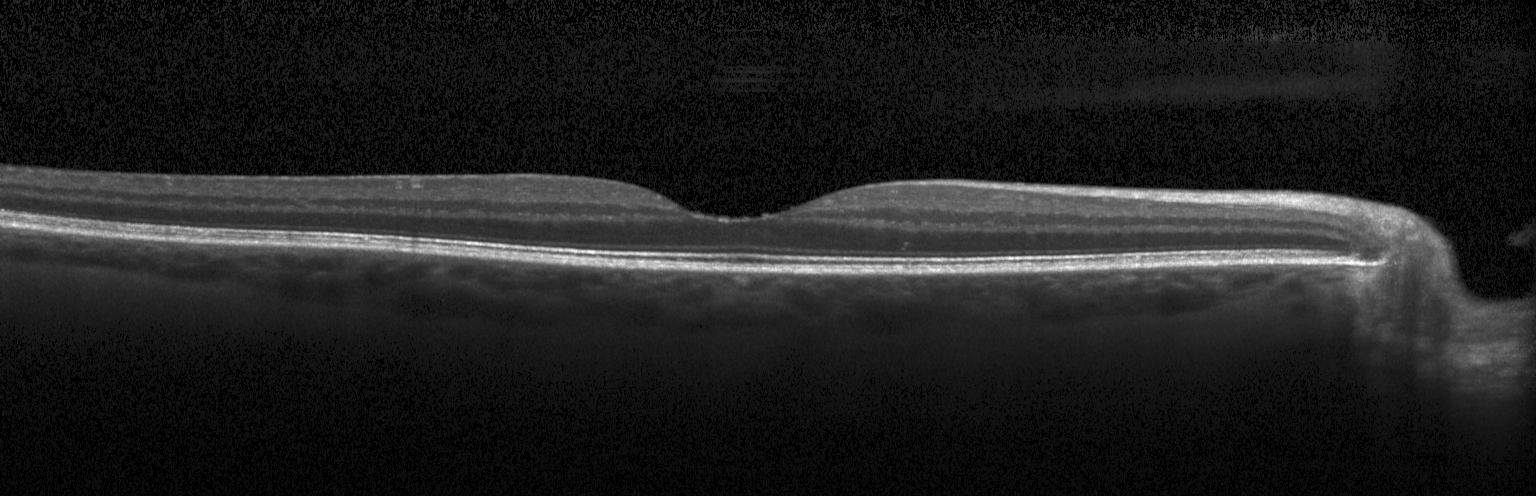 Retinal OCT cross-section
Finding: neither choroidal neovascularization, diabetic macular edema, nor drusen.